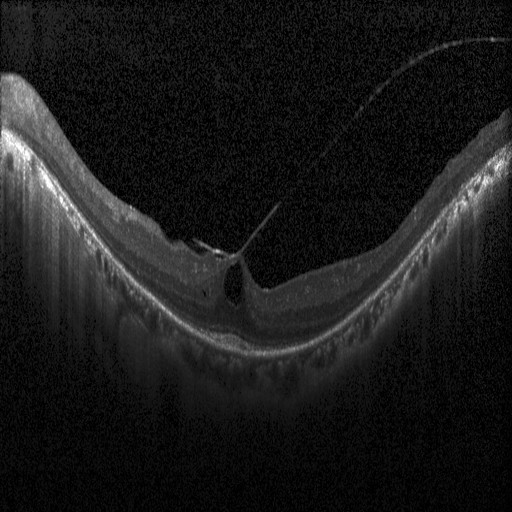 OCT B-scan
Diabetic macular edema (DME).